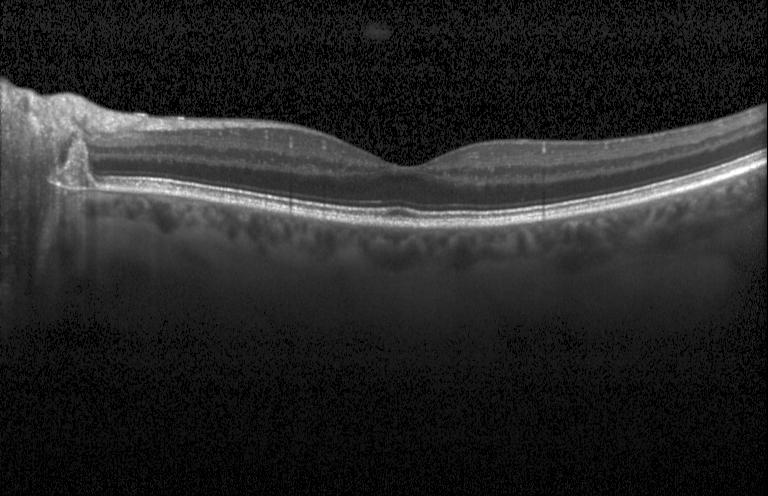 SD-OCT; Heidelberg Spectralis; centered on the fovea; retinal OCT cross-section. Assessment: no choroidal neovascularization, diabetic macular edema, or drusen.